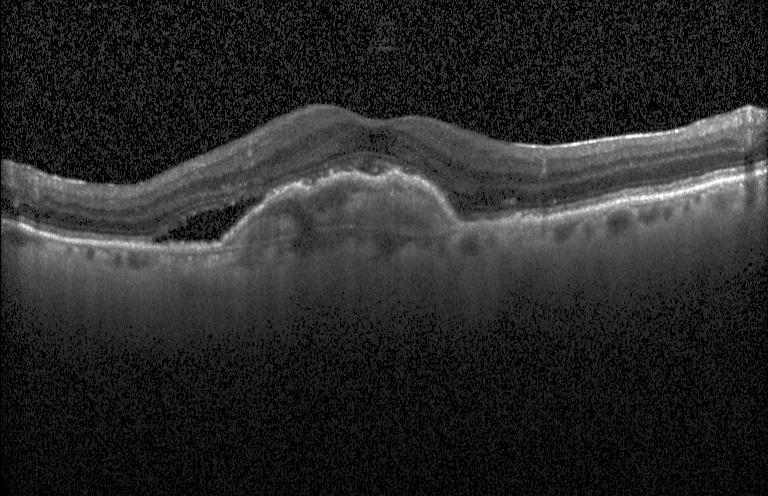

Spectral-domain optical coherence tomography. Optical coherence tomography B-scan. Through the macula. Diagnosis: a choroidal neovascular membrane.